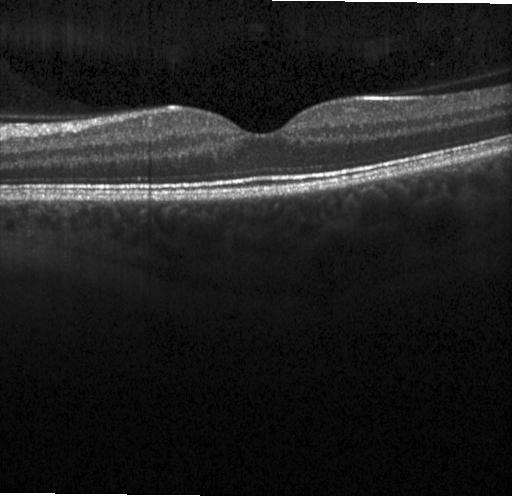 Impression: no choroidal neovascularization, no diabetic macular edema, and no drusen.